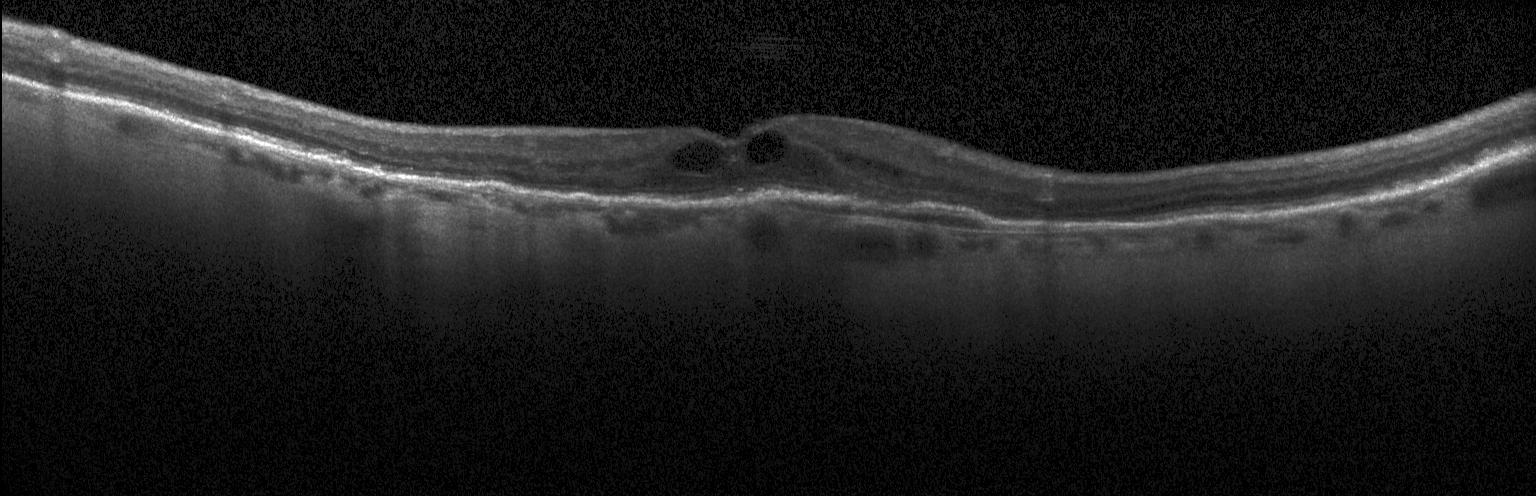 Fovea-centered; Heidelberg Spectralis; SD-OCT; OCT line scan.
This B-scan demonstrates CNV.